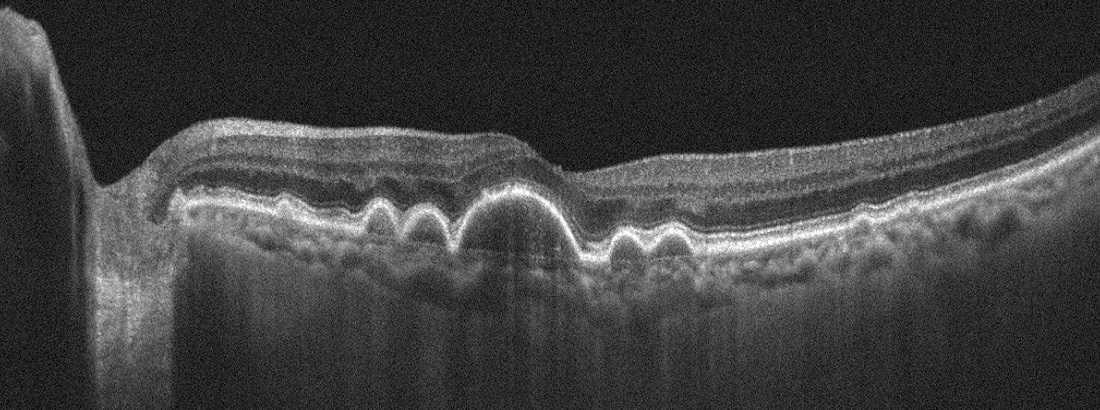 Acquired on an Optovue Avanti RTVue XR · optical coherence tomography scan.
OCT finding: AMD.